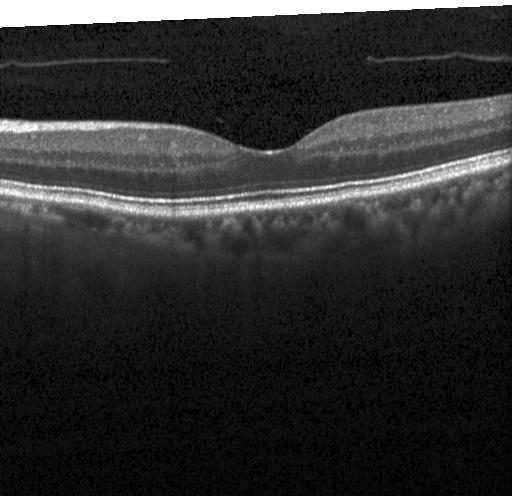 Retinal OCT cross-section showing no choroidal neovascularization, diabetic macular edema, or drusen.